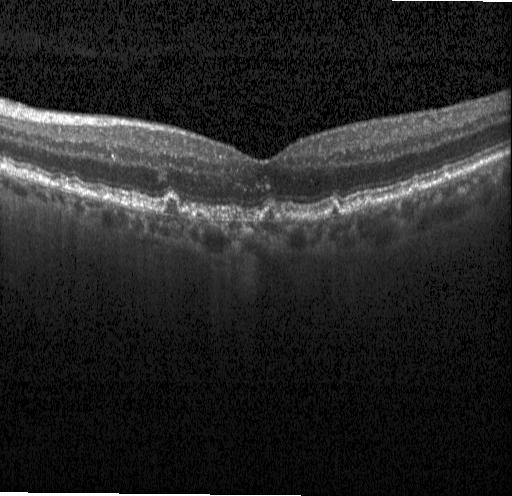 Finding: drusen.